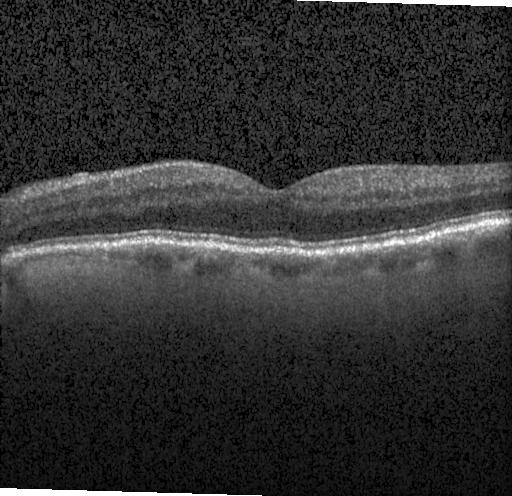 The scan shows no choroidal neovascularization, diabetic macular edema, or drusen.